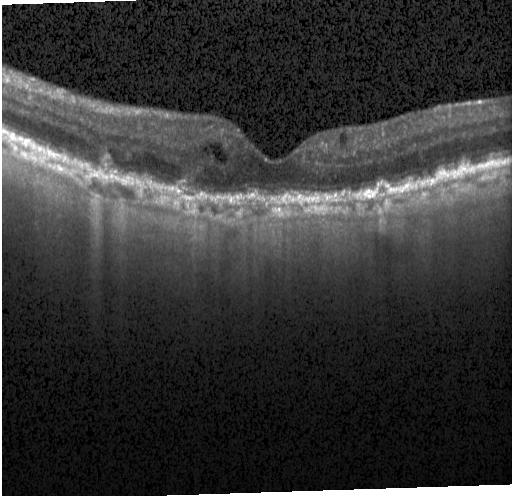 Impression: choroidal neovascularization (CNV).